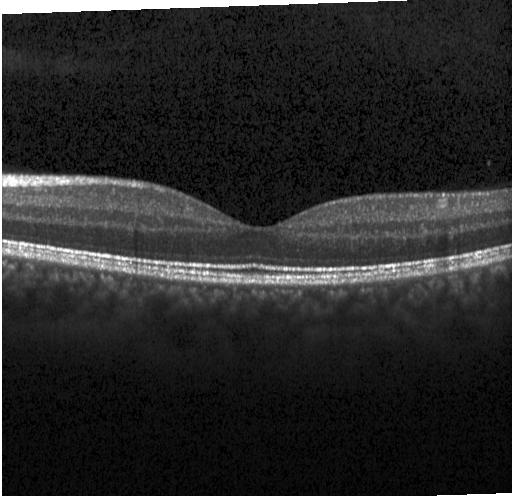 OCT B-scan showing neither CNV, DME, nor drusen.